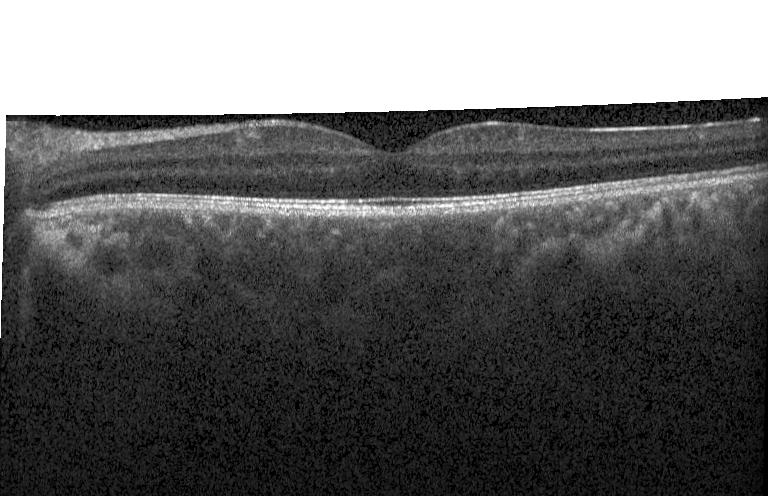
Macular OCT: no CNV, no DME, and no drusen.